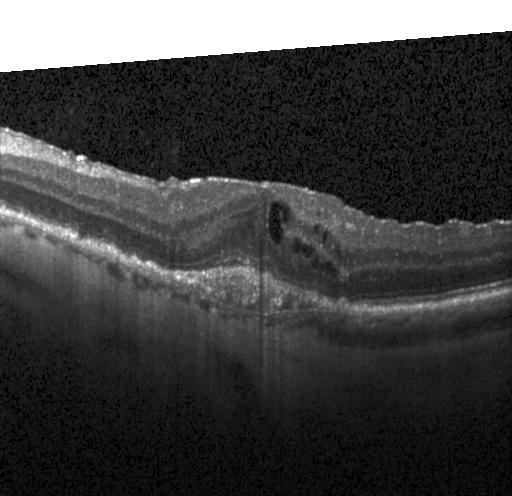
Acquired on a Heidelberg Spectralis · optical coherence tomography B-scan. Dx: a choroidal neovascular membrane.